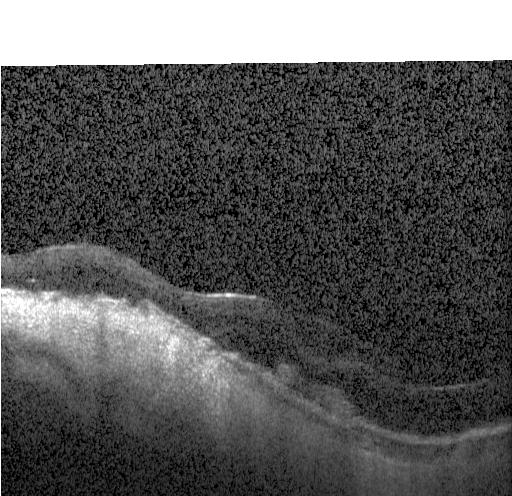
OCT B-scan. Assessment: CNV.